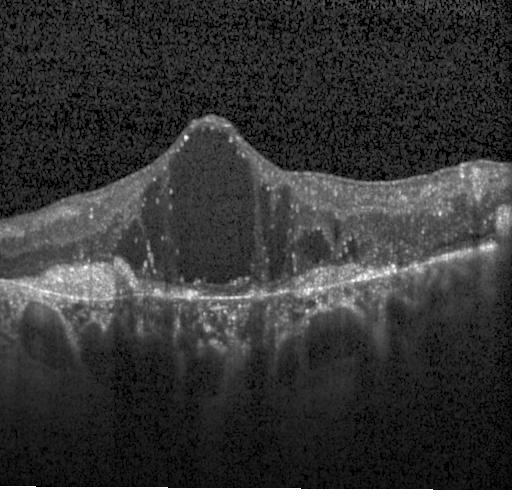 Spectral-domain OCT · Heidelberg Spectralis · horizontal scan through the fovea · optical coherence tomography scan.
Diagnosis: choroidal neovascularization.